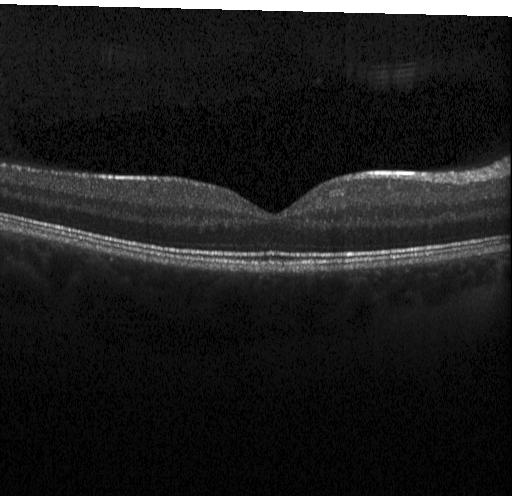 OCT finding: no choroidal neovascularization, no diabetic macular edema, and no drusen.